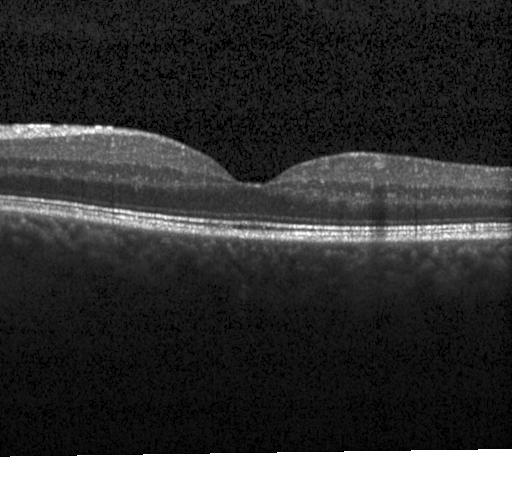 Impression: neither CNV, DME, nor drusen.